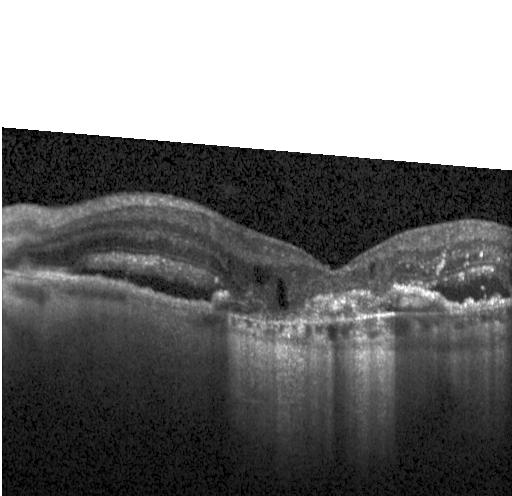

OCT line scan · horizontal scan through the fovea.
Assessment: a choroidal neovascular membrane.